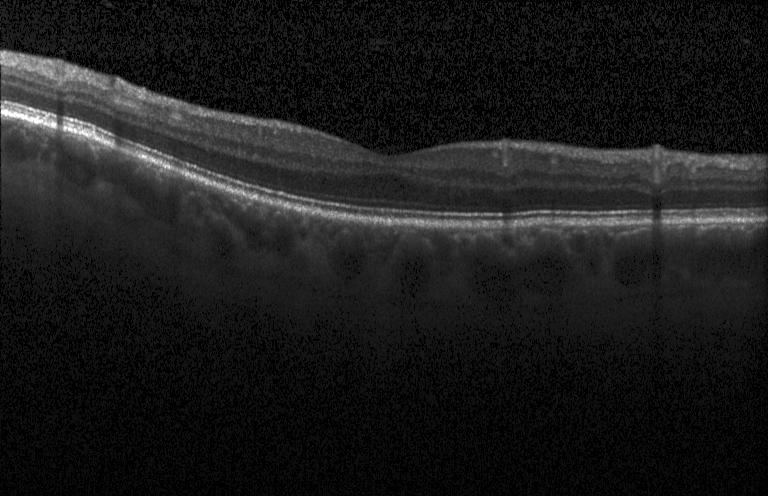 OCT finding: neither choroidal neovascularization, diabetic macular edema, nor drusen.